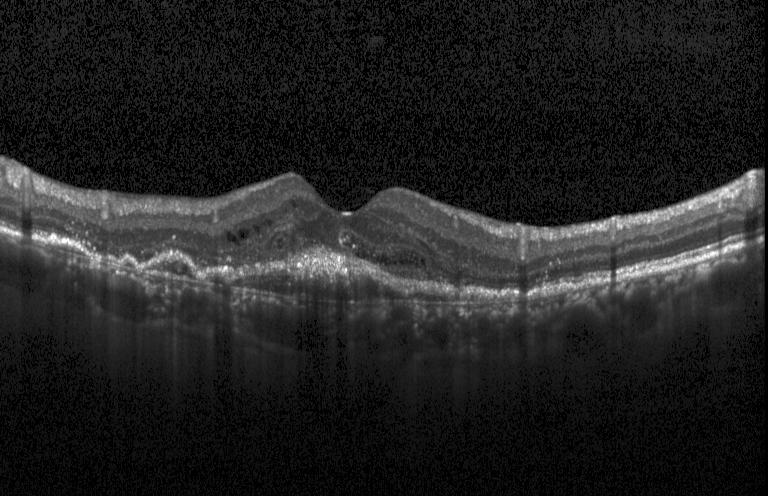
Retinal OCT B-scan · through the macula · Heidelberg Spectralis · spectral-domain optical coherence tomography. A choroidal neovascular membrane.